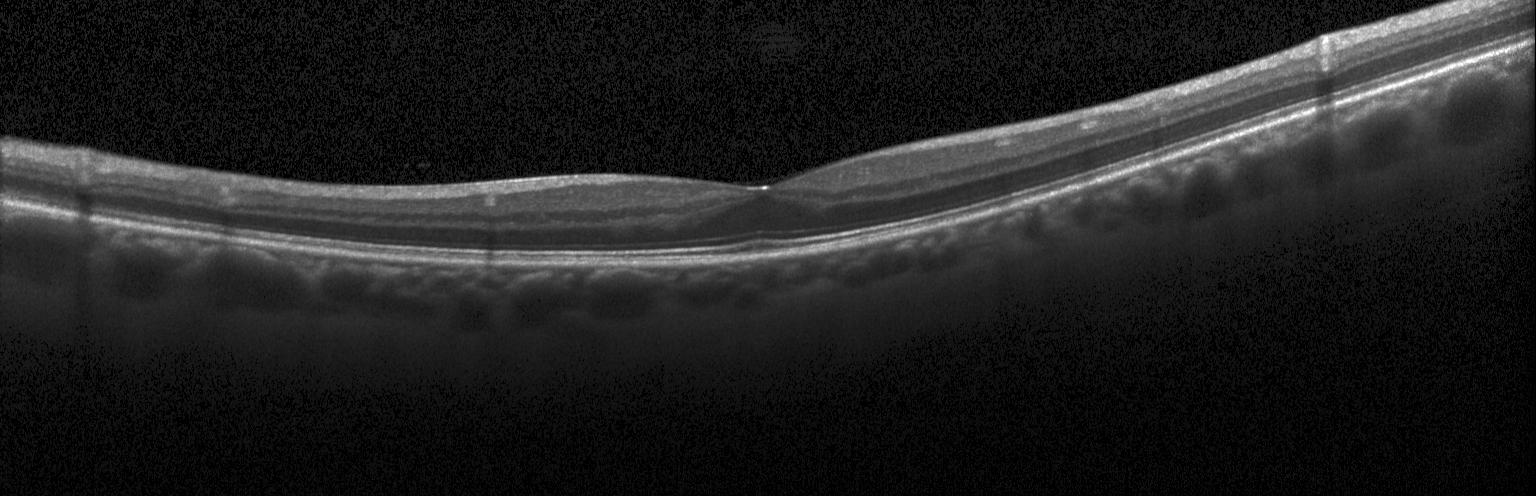

Fovea-centered, SD-OCT, OCT B-scan, acquired on a Heidelberg Spectralis. Diagnosis: neither choroidal neovascularization, diabetic macular edema, nor drusen.